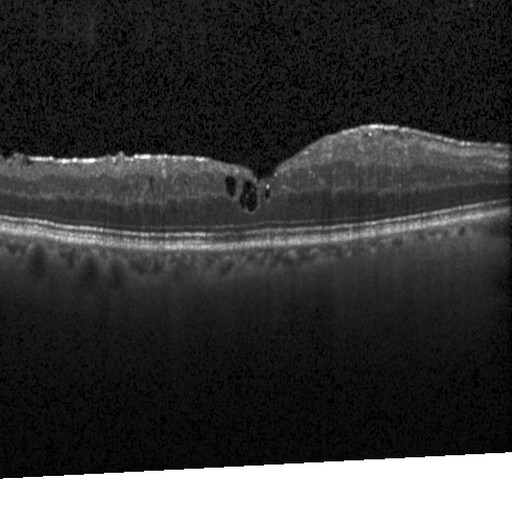 Retinal OCT cross-section showing diabetic macular edema.